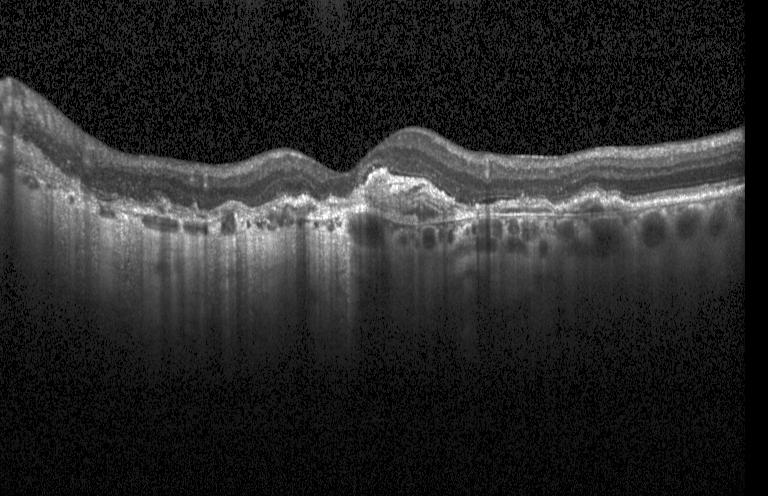 Finding: choroidal neovascularization (CNV).